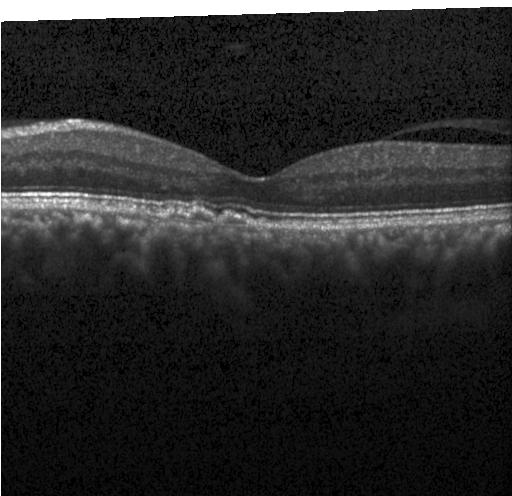

Assessment: sub-RPE drusenoid deposits.